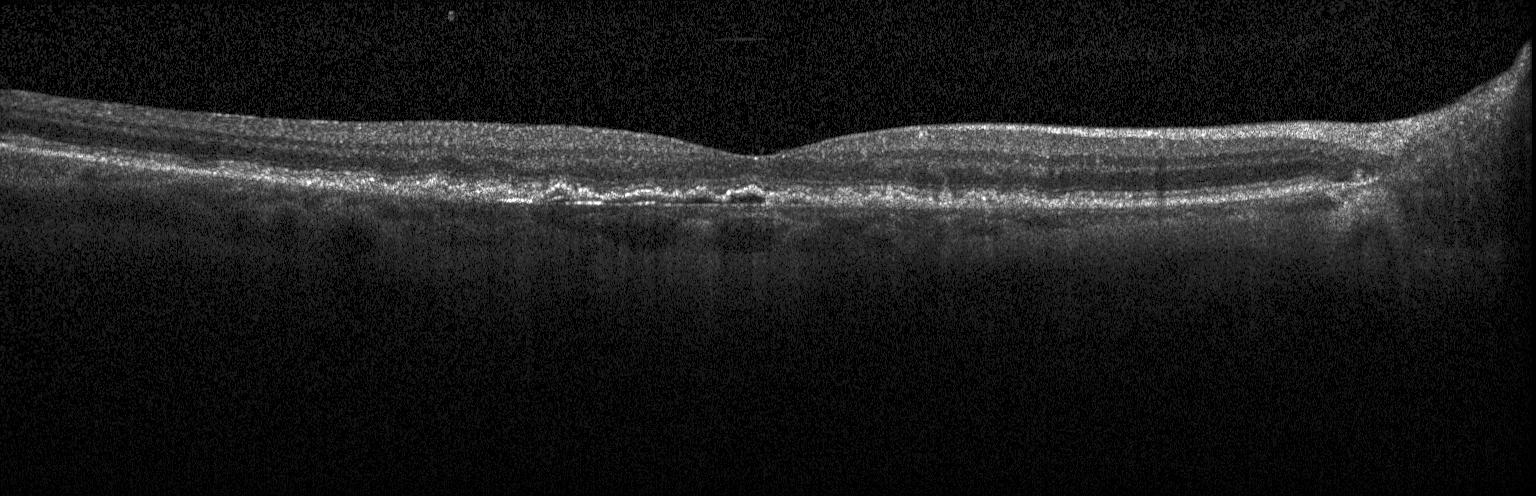 Spectral-domain OCT B-scan: choroidal neovascularization (CNV).